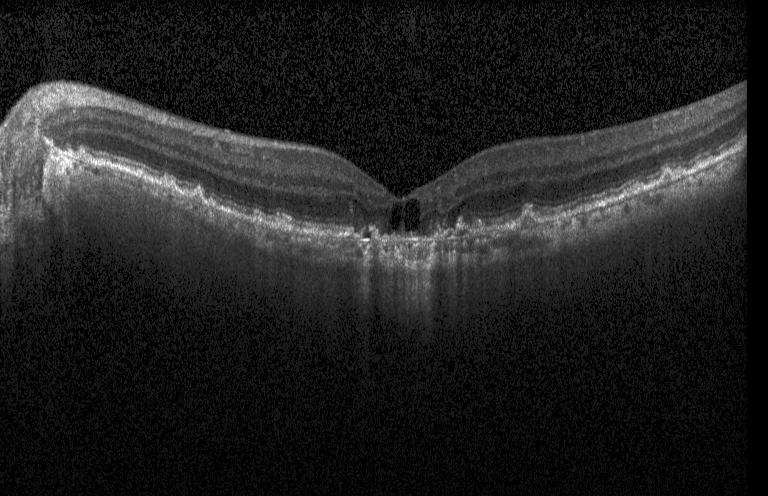
Optical coherence tomography B-scan · Heidelberg Spectralis · fovea-centered
The scan shows CNV.